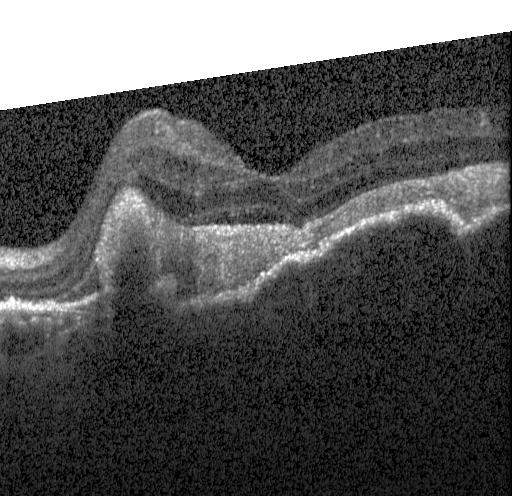

Retinal OCT cross-section showing choroidal neovascularization.